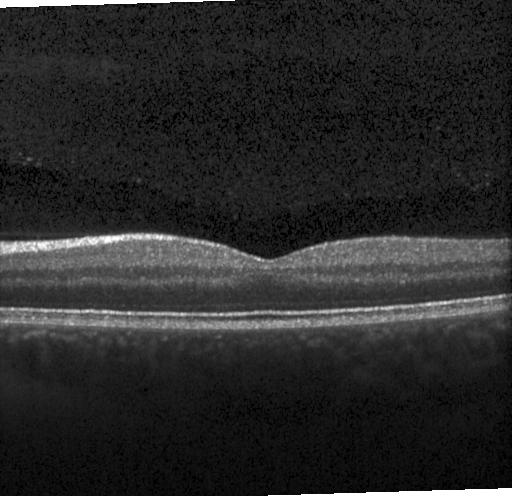 Optical coherence tomography B-scan.
OCT finding: no choroidal neovascularization, no diabetic macular edema, and no drusen.